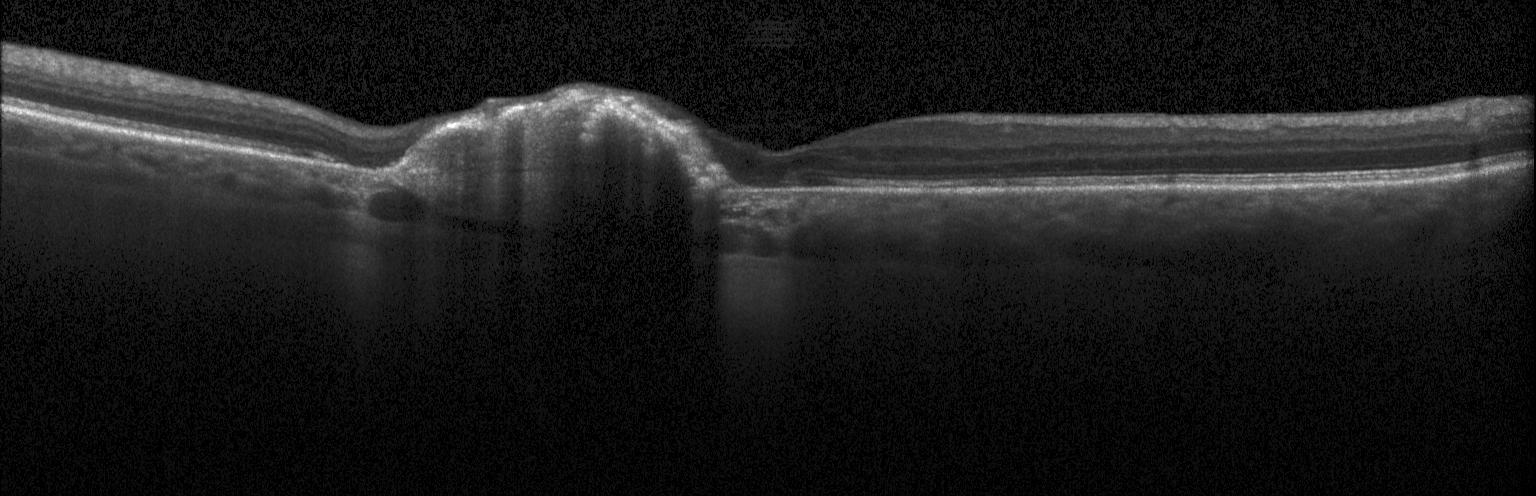

OCT line scan.
This B-scan demonstrates CNV.